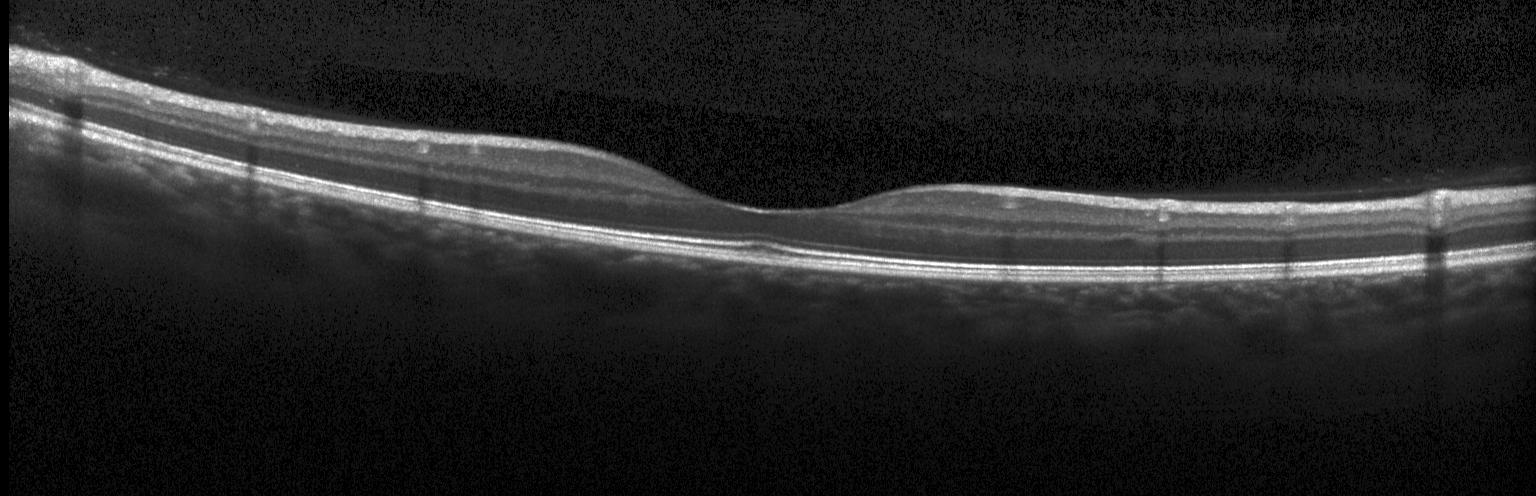 OCT finding: neither choroidal neovascularization, diabetic macular edema, nor drusen.